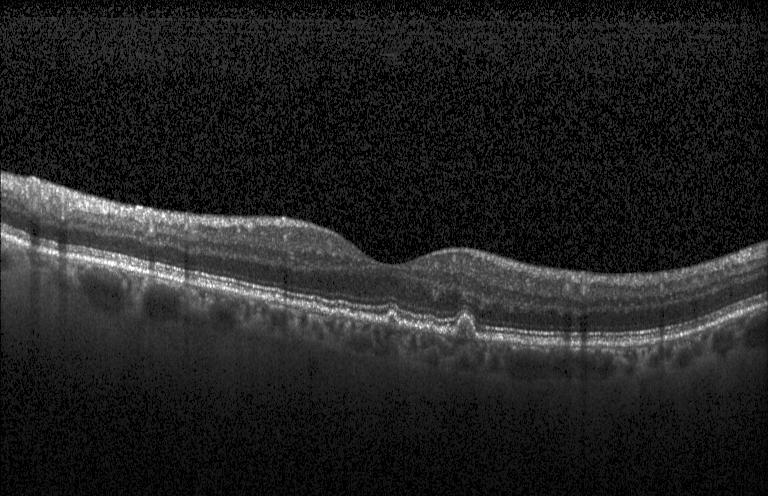
OCT finding: multiple drusen.